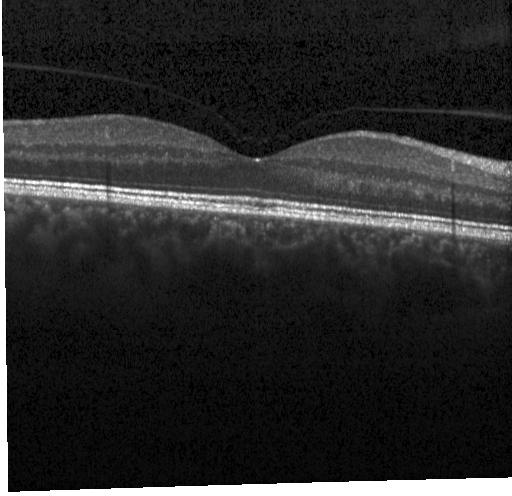
This B-scan demonstrates no choroidal neovascularization, diabetic macular edema, or drusen.